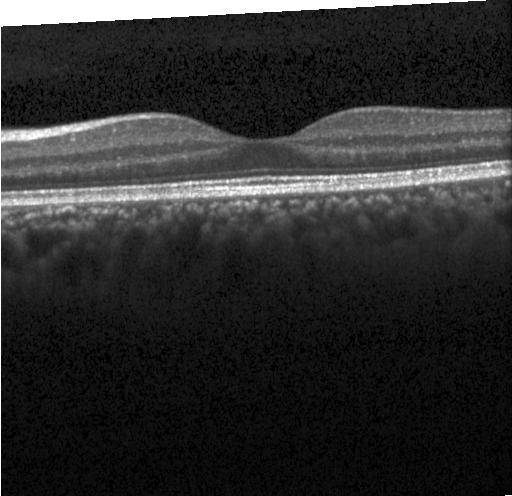 OCT line scan, horizontal scan through the fovea. Diagnosis: no choroidal neovascularization, no diabetic macular edema, and no drusen.